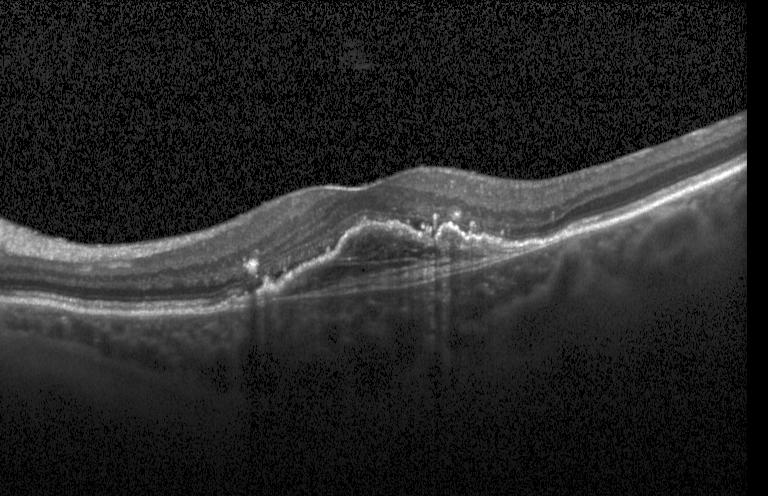

Retinal OCT cross-section showing a choroidal neovascular membrane.